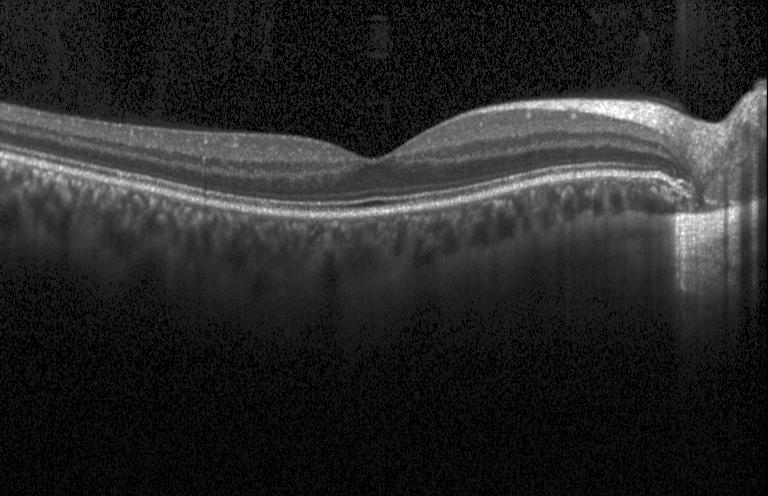
Optical coherence tomography B-scan.
Dx: neither CNV, DME, nor drusen.